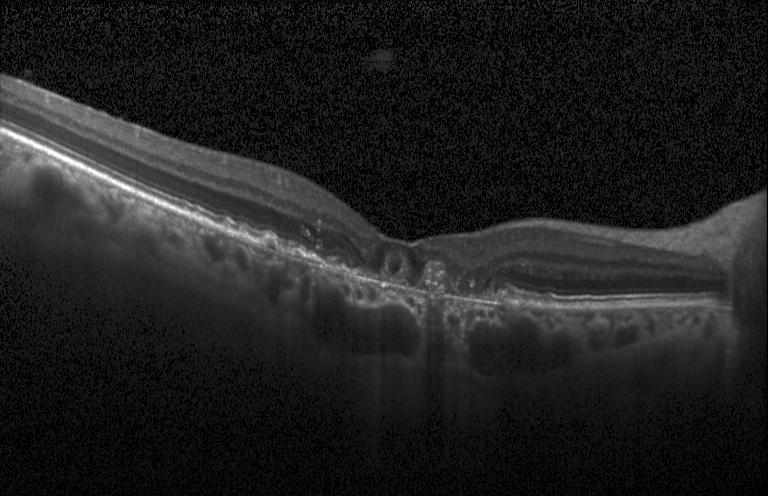
Heidelberg Spectralis. Through the macula. Optical coherence tomography B-scan. Spectral-domain optical coherence tomography. Assessment: choroidal neovascularization (CNV).